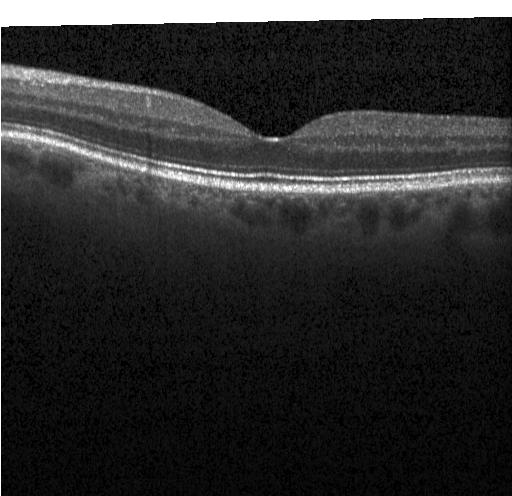 Dx: neither choroidal neovascularization, diabetic macular edema, nor drusen.